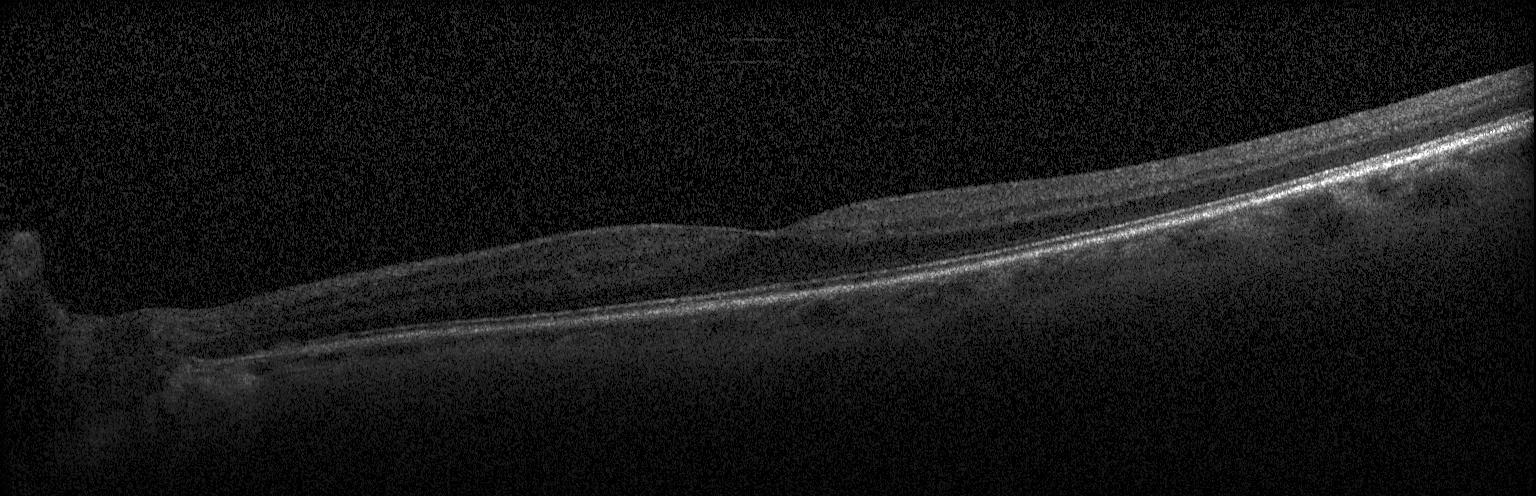
Heidelberg Spectralis, retinal OCT B-scan.
Finding: no choroidal neovascularization, diabetic macular edema, or drusen.